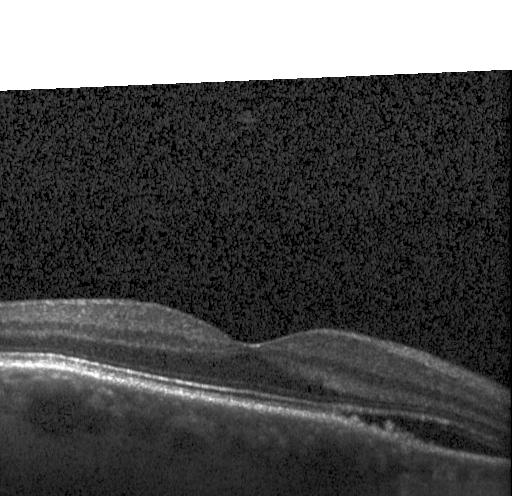 OCT line scan
Impression: a choroidal neovascular membrane.